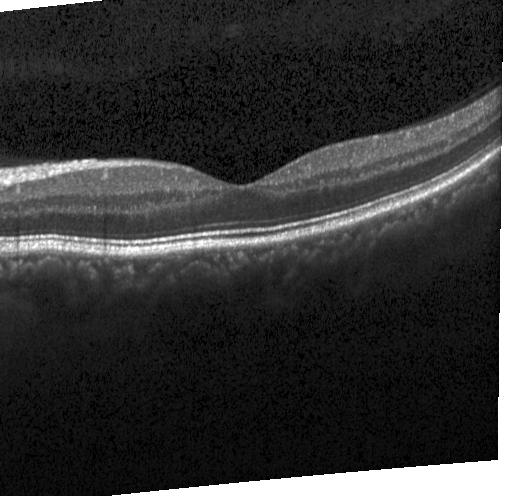 Impression: neither CNV, DME, nor drusen.